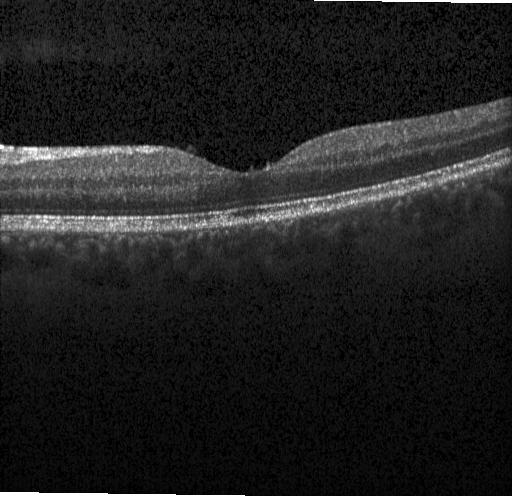 Macular scan, instrument: Heidelberg Spectralis, spectral-domain OCT, OCT B-scan
This B-scan demonstrates neither choroidal neovascularization, diabetic macular edema, nor drusen.